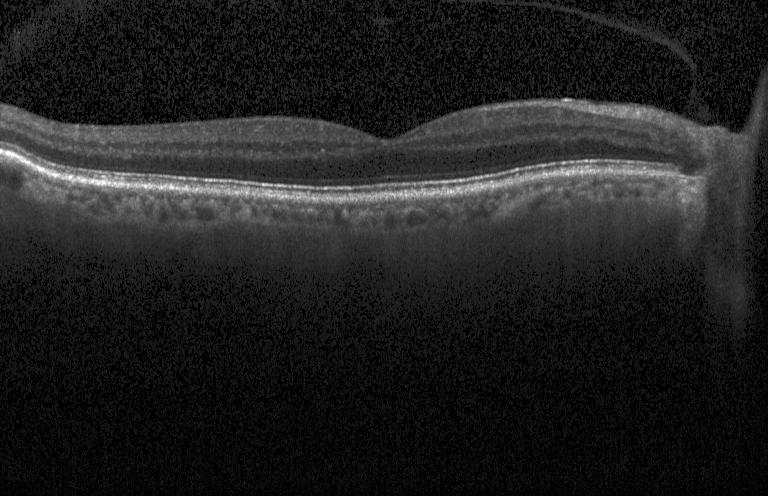
Centered on the fovea · Heidelberg Spectralis · OCT line scan — Dx: no CNV, no DME, and no drusen.